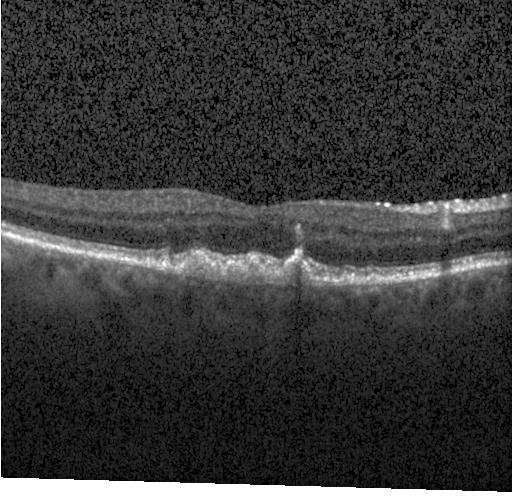

Finding: sub-RPE drusenoid deposits.